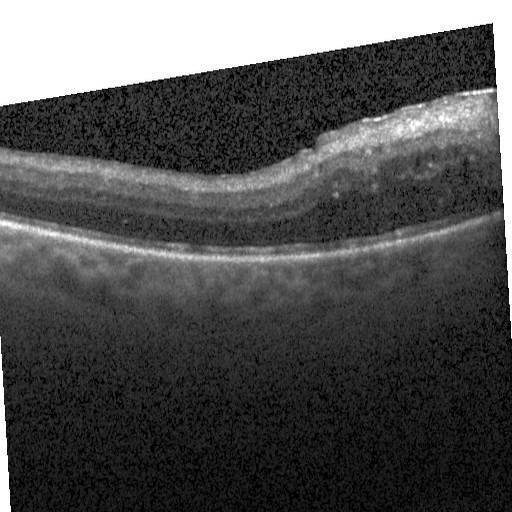
Heidelberg Spectralis. Through the macula. Optical coherence tomography scan — Diagnosis: DME.